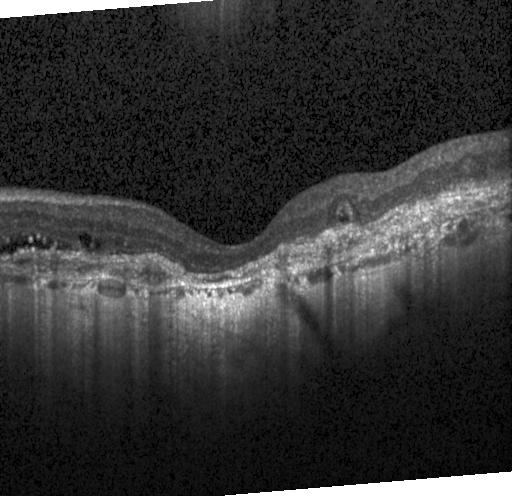 Macular OCT demonstrating a choroidal neovascular membrane.